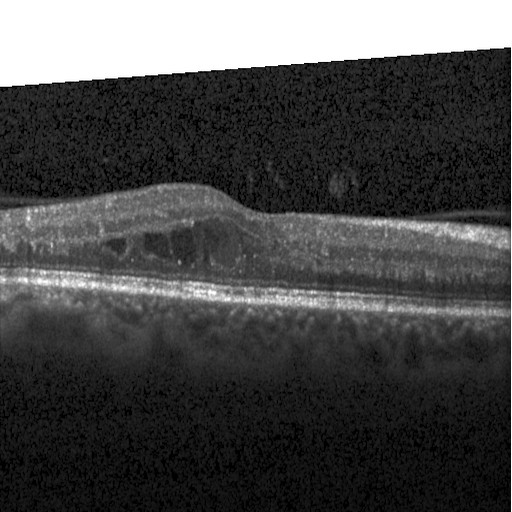

Optical coherence tomography scan — Assessment: diabetic macular edema (DME).